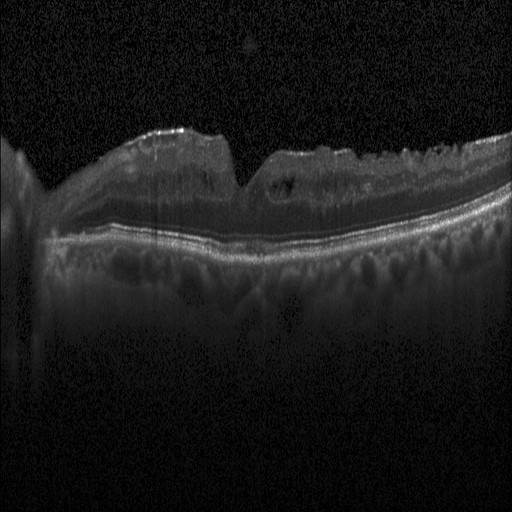

OCT line scan; through the macula; spectral-domain OCT. Impression: DME.